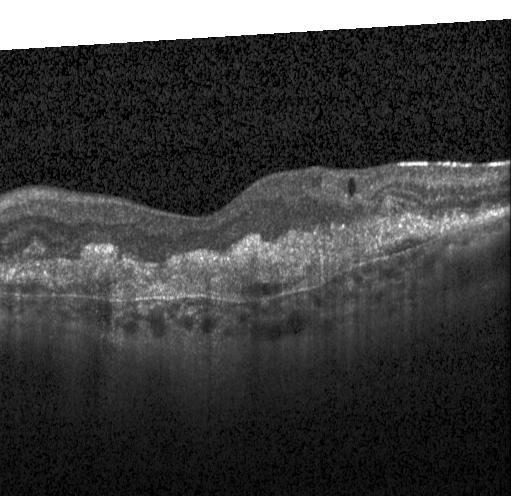

Spectral-domain optical coherence tomography · Heidelberg Spectralis · retinal OCT B-scan · through the macula — Assessment: choroidal neovascularization.